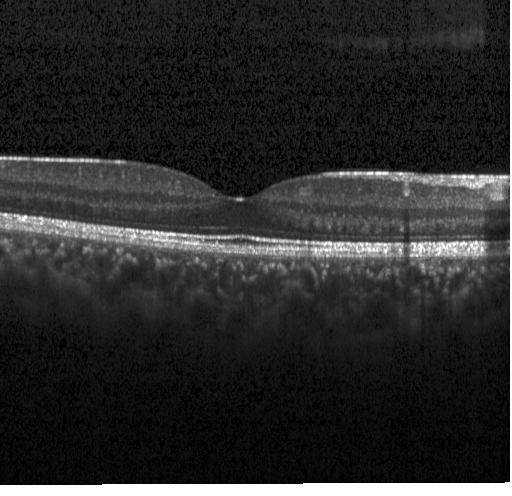 Instrument: Heidelberg Spectralis · through the macula · OCT line scan · spectral-domain OCT.
Finding: no choroidal neovascularization, diabetic macular edema, or drusen.